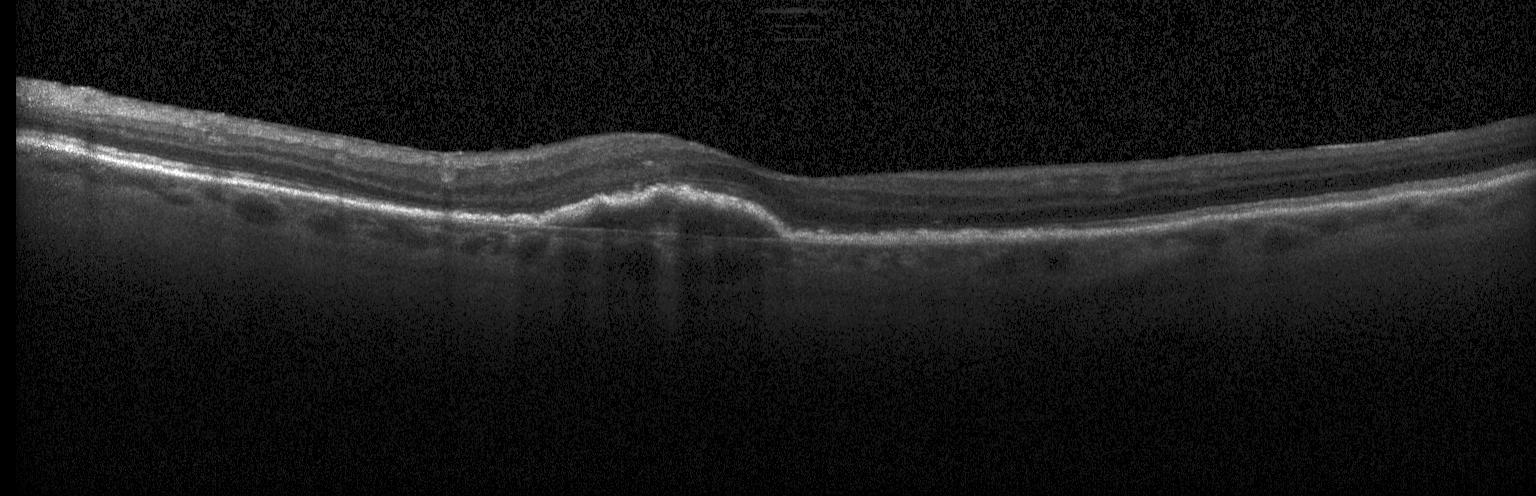 Fovea-centered; acquired on a Heidelberg Spectralis; OCT line scan — Diagnosis: choroidal neovascularization (CNV).